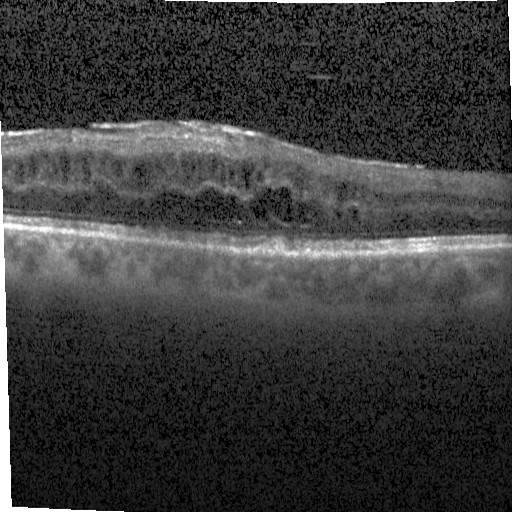
Impression: diabetic macular edema.